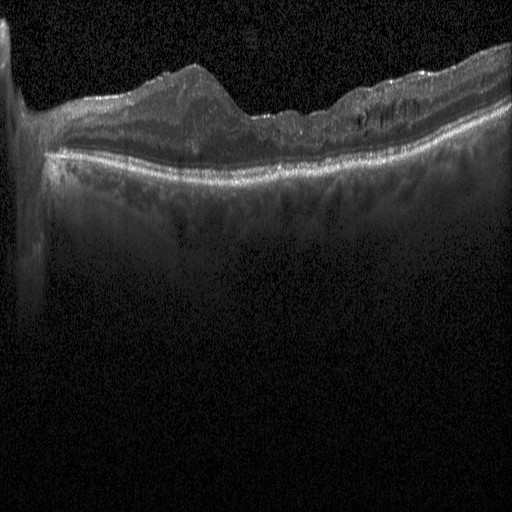
OCT B-scan.
The scan shows diabetic macular edema.